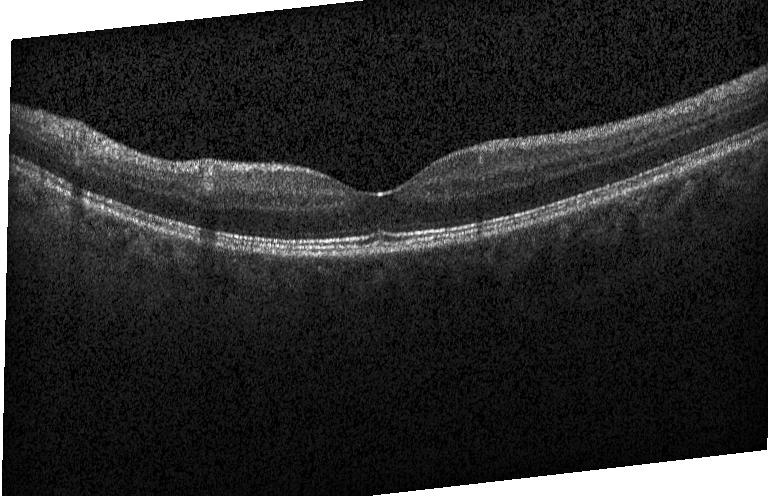
Impression: no choroidal neovascularization, diabetic macular edema, or drusen.